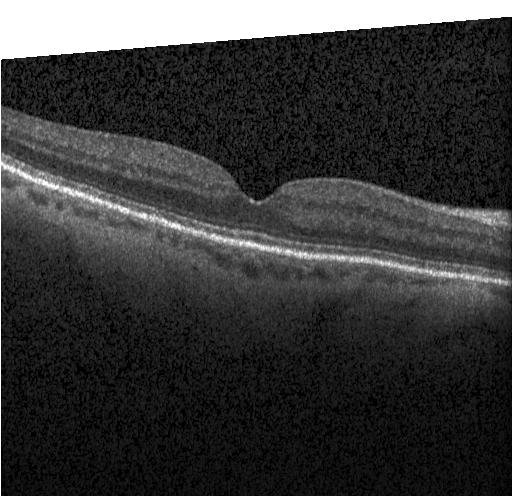

Optical coherence tomography scan · SD-OCT · fovea-centered. The scan shows neither choroidal neovascularization, diabetic macular edema, nor drusen.